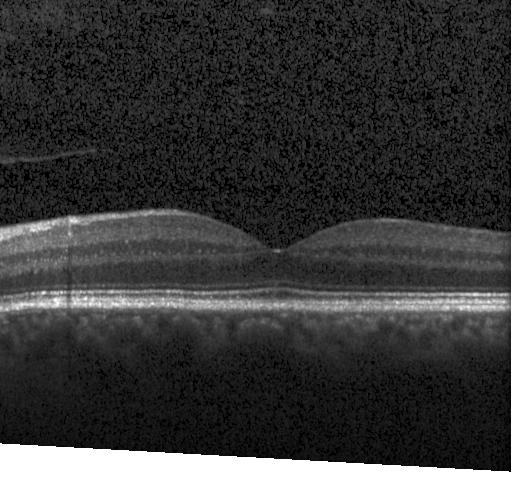
OCT B-scan; acquired on a Heidelberg Spectralis — The scan shows no choroidal neovascularization, diabetic macular edema, or drusen.